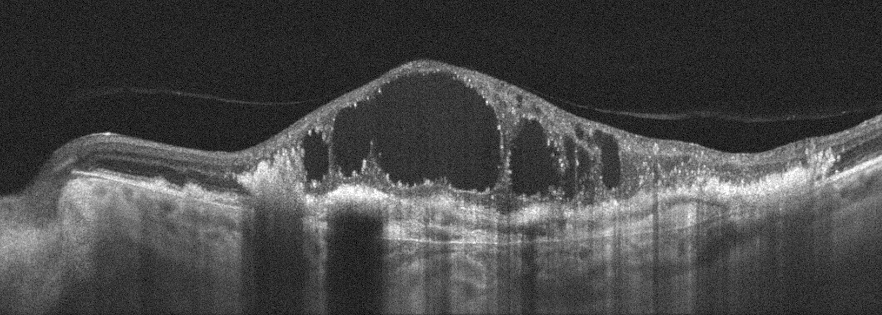

Left eye. Retinal OCT cross-section.
Impression: AMD.